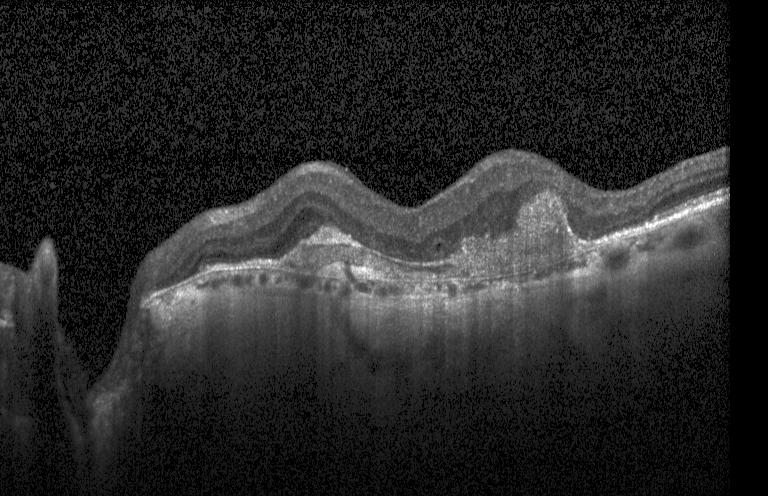
Impression: a choroidal neovascular membrane.